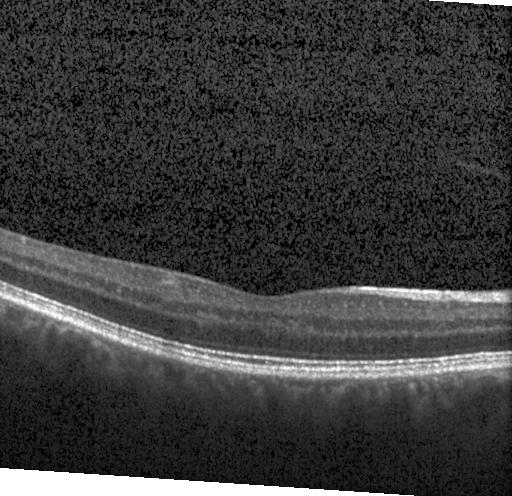 Retinal OCT B-scan, Heidelberg Spectralis OCT system
Diagnosis: no choroidal neovascularization, no diabetic macular edema, and no drusen.